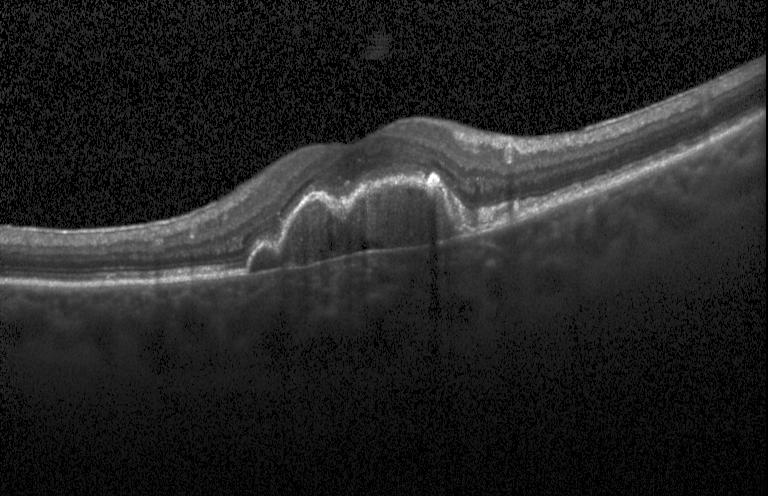

Macular OCT demonstrating a choroidal neovascular membrane.